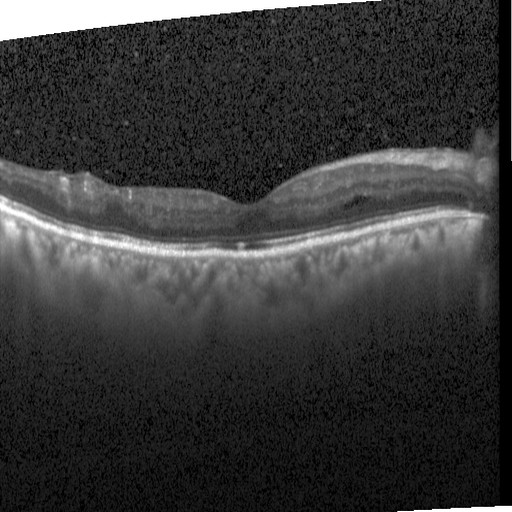 Retinal OCT cross-section showing diabetic macular edema.